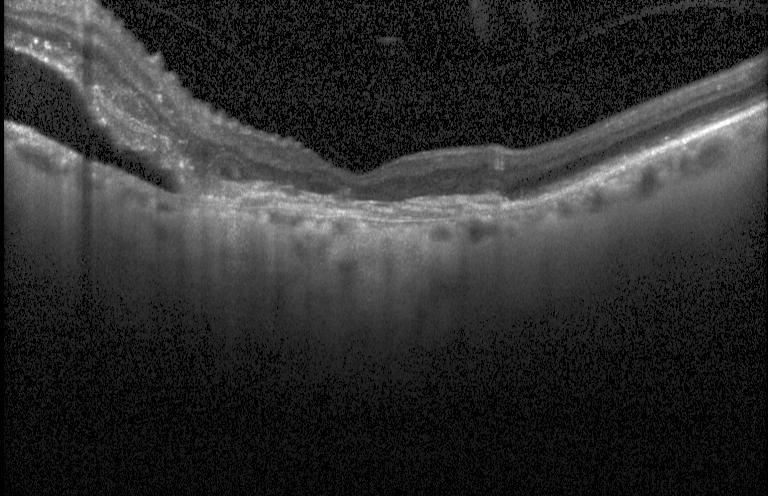

Finding: choroidal neovascularization (CNV).